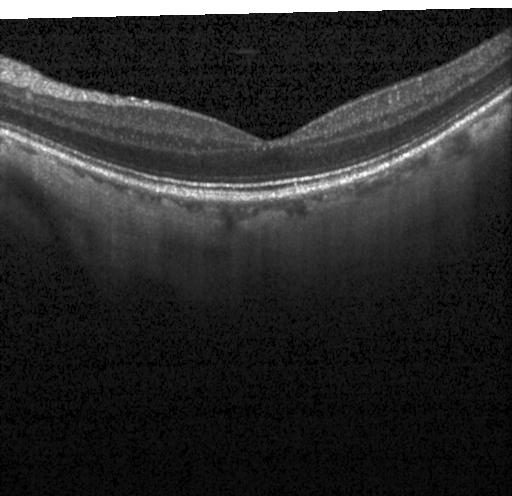
Spectral-domain optical coherence tomography; optical coherence tomography scan — Impression: neither CNV, DME, nor drusen.